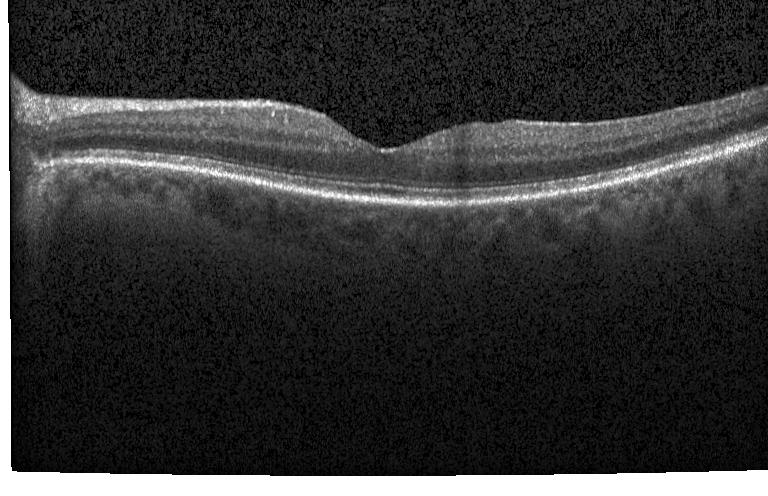

Macular OCT demonstrating no evidence of choroidal neovascularization, diabetic macular edema, or drusen.